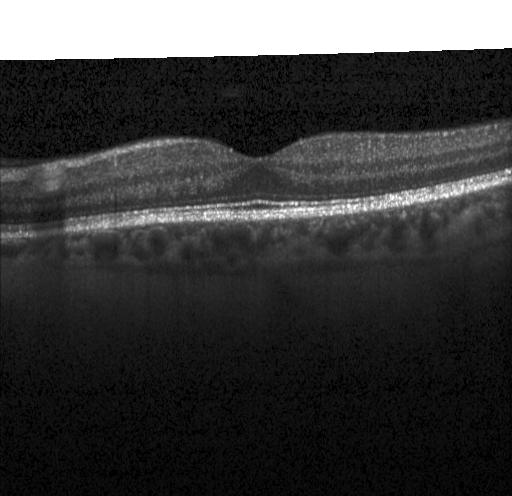

Impression: no choroidal neovascularization, diabetic macular edema, or drusen.